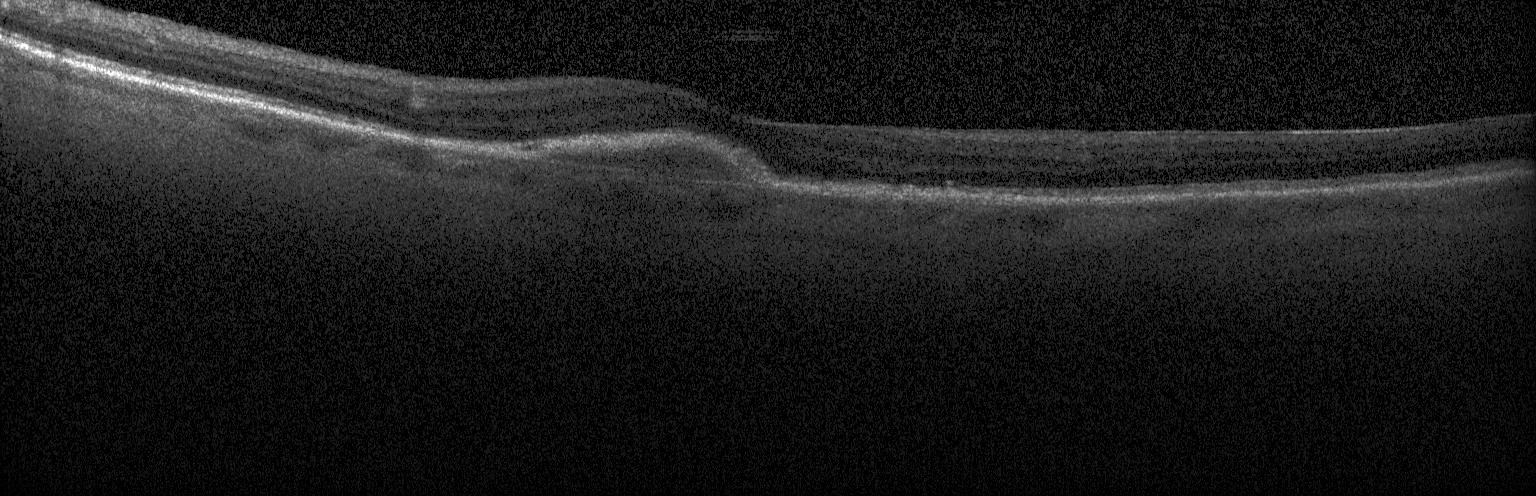 Macular OCT: CNV.